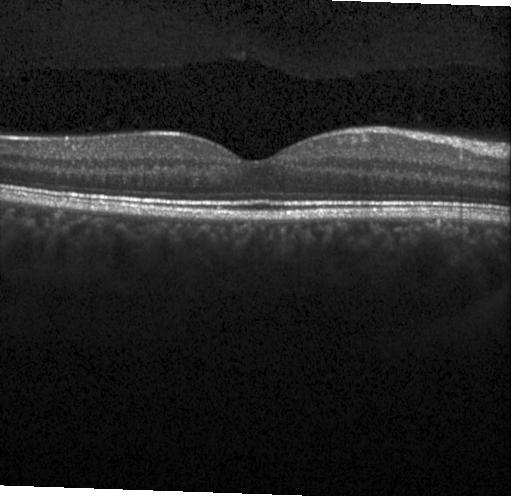 Optical coherence tomography B-scan. Impression: no evidence of choroidal neovascularization, diabetic macular edema, or drusen.